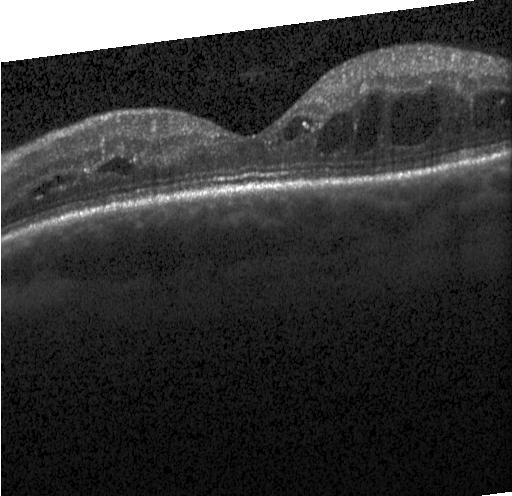 Macular OCT: diabetic macular edema (DME).